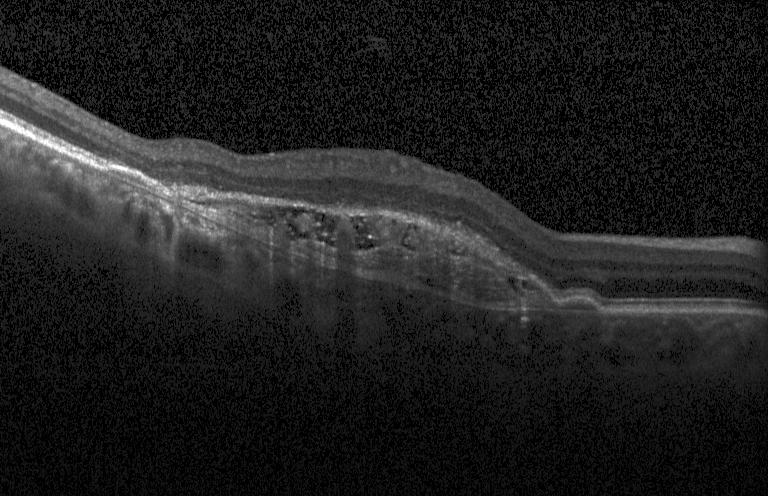 Heidelberg Spectralis OCT system. Through the macula. OCT B-scan
Impression: a choroidal neovascular membrane.